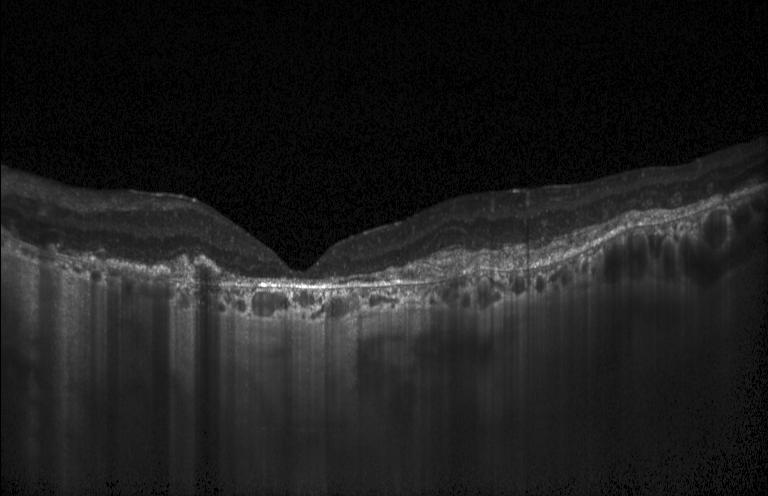

Macular OCT: choroidal neovascularization.